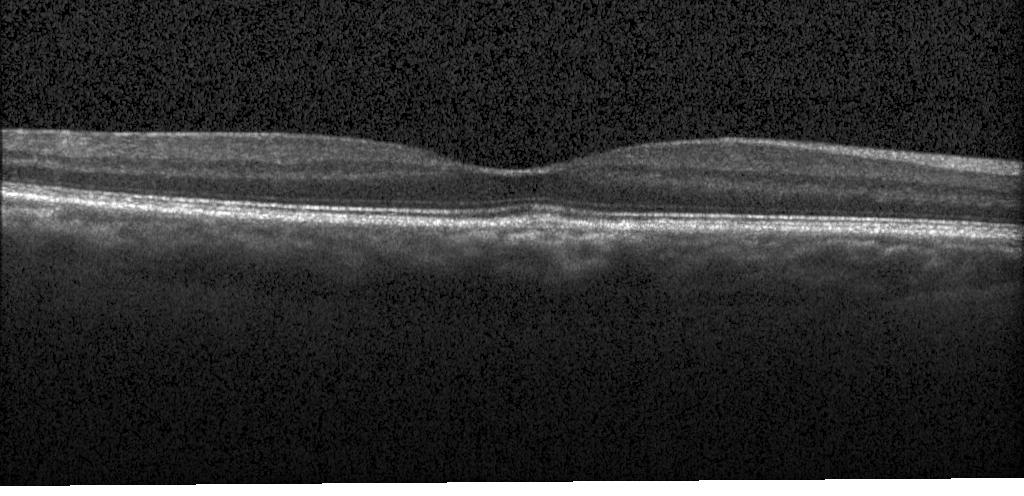

Diagnosis: no choroidal neovascularization, diabetic macular edema, or drusen.